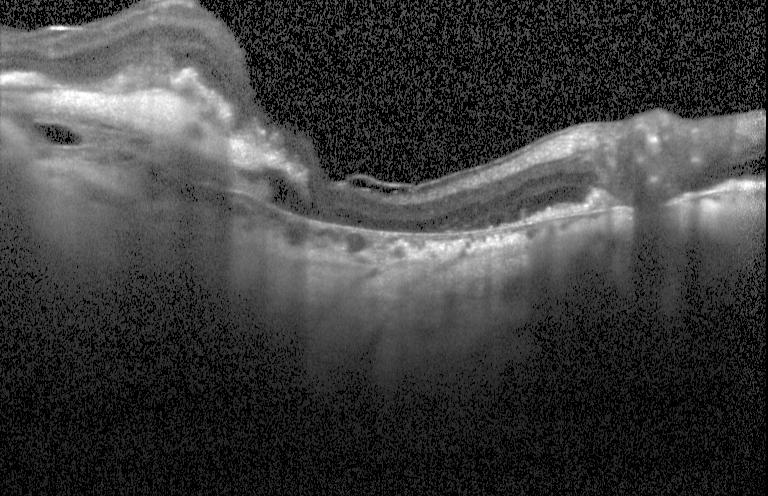

Optical coherence tomography B-scan.
Impression: a choroidal neovascular membrane.